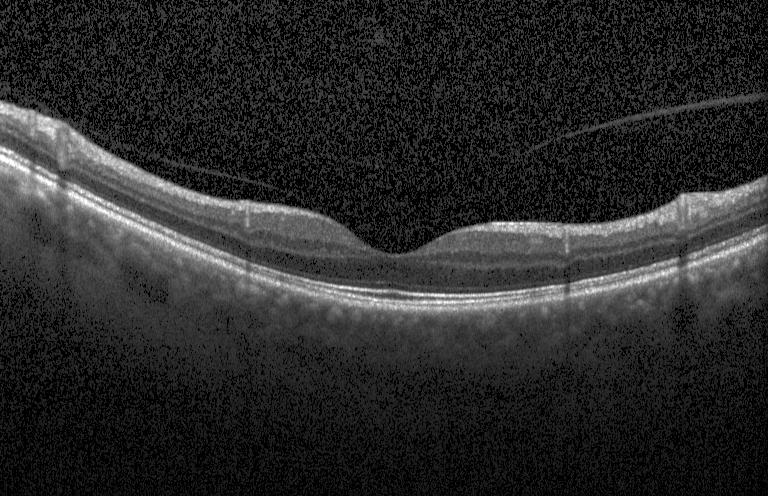

Fovea-centered; acquired on a Heidelberg Spectralis; OCT line scan; SD-OCT.
Dx: no evidence of choroidal neovascularization, diabetic macular edema, or drusen.